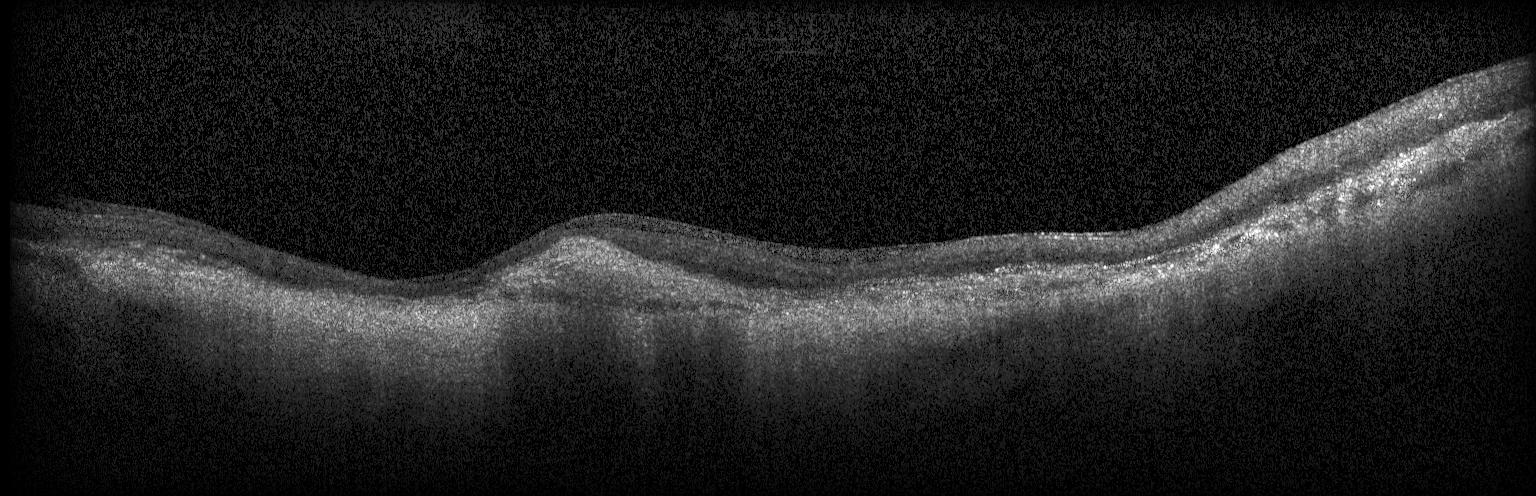 Spectral-domain OCT, fovea-centered, optical coherence tomography B-scan — Dx: CNV.